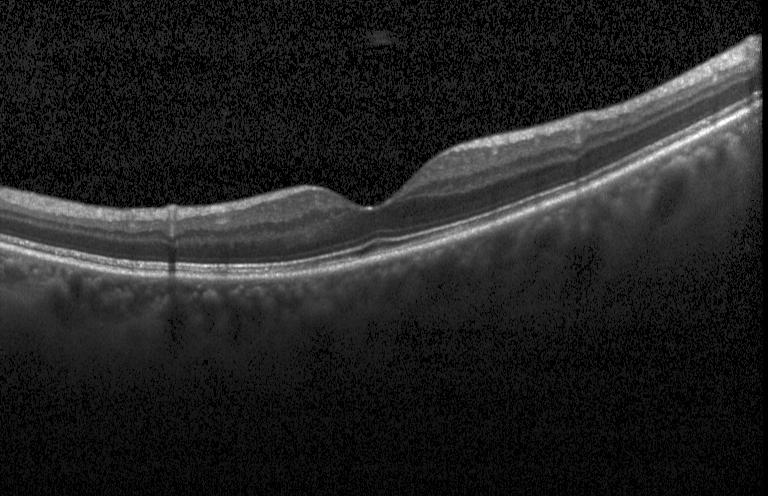

Horizontal scan through the fovea, optical coherence tomography scan
Diagnosis: no choroidal neovascularization, diabetic macular edema, or drusen.